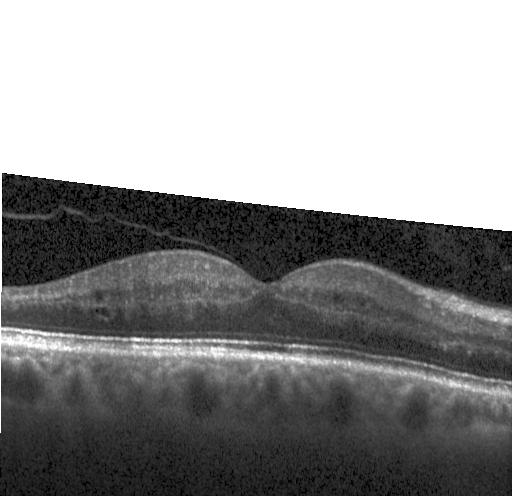 Optical coherence tomography scan. The scan shows diabetic macular edema (DME).